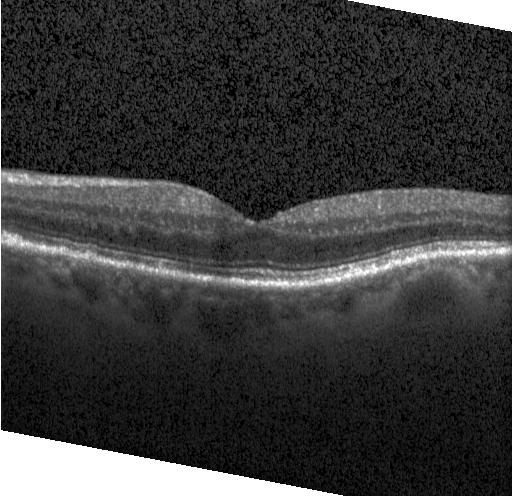 Fovea-centered · OCT B-scan · spectral-domain OCT.
Neither choroidal neovascularization, diabetic macular edema, nor drusen.